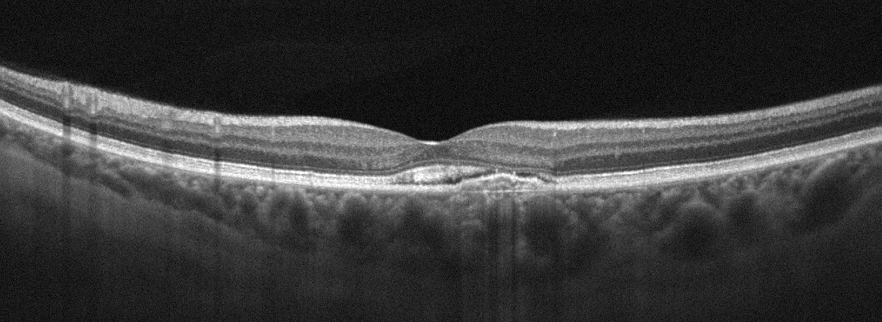
Oculus sinister, retinal OCT cross-section
Finding: age-related macular degeneration.